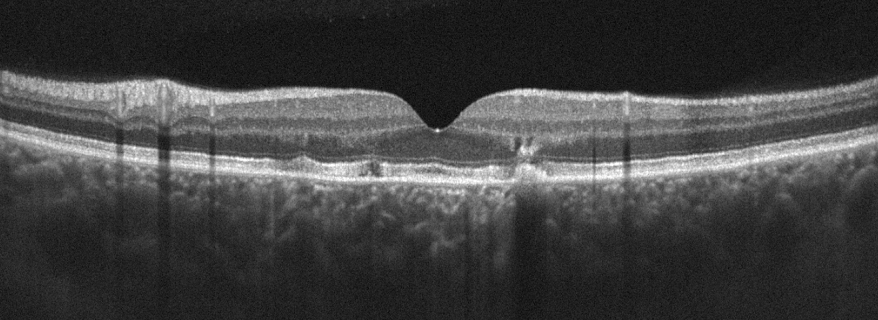
OCT B-scan showing AMD.